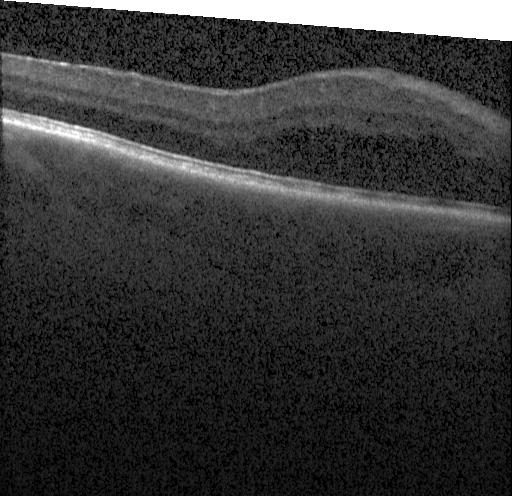 OCT finding: DME.